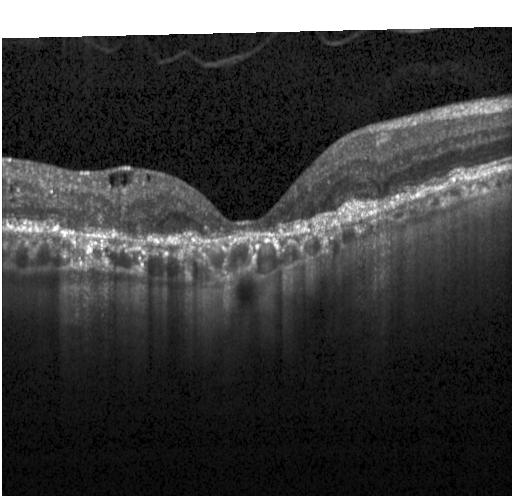
OCT finding: a choroidal neovascular membrane.